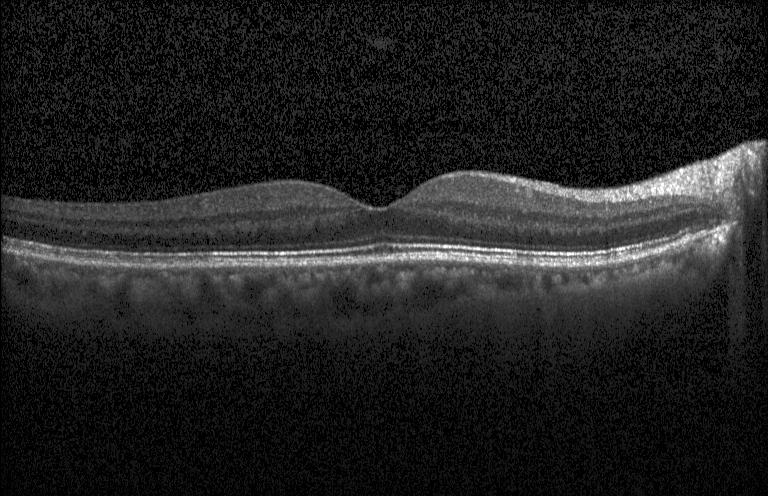
Retinal OCT cross-section. Macular scan. Spectral-domain optical coherence tomography. Instrument: Heidelberg Spectralis. No evidence of choroidal neovascularization, diabetic macular edema, or drusen.